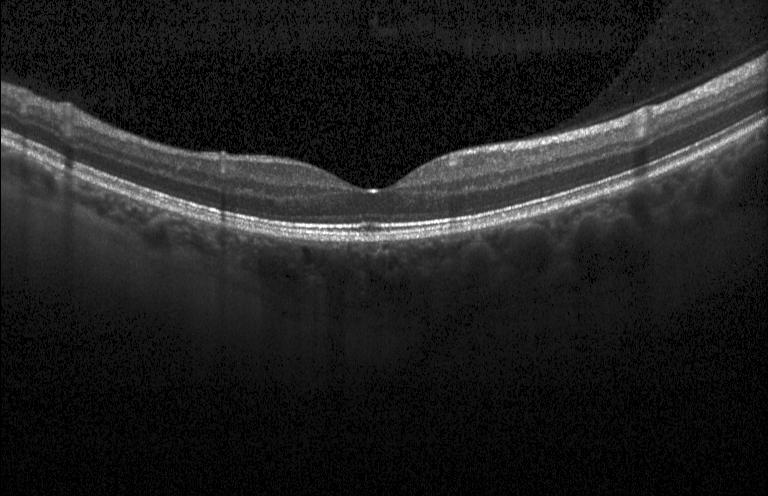
OCT B-scan. OCT finding: neither CNV, DME, nor drusen.